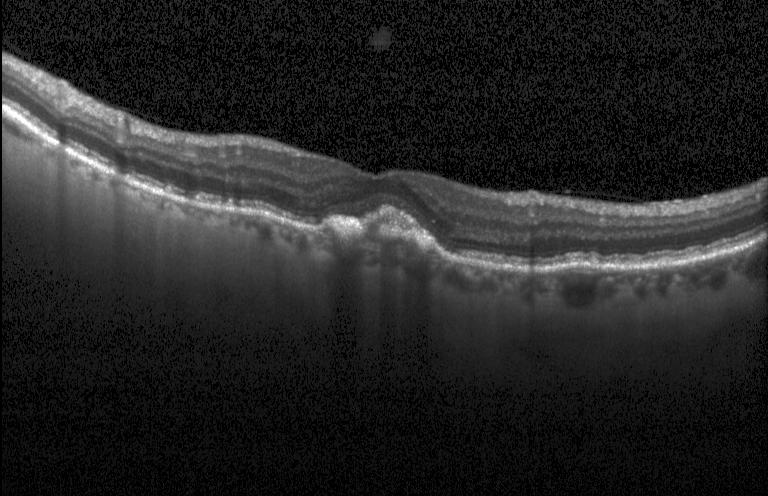
Centered on the fovea. Retinal OCT B-scan. Diagnosis: choroidal neovascularization.